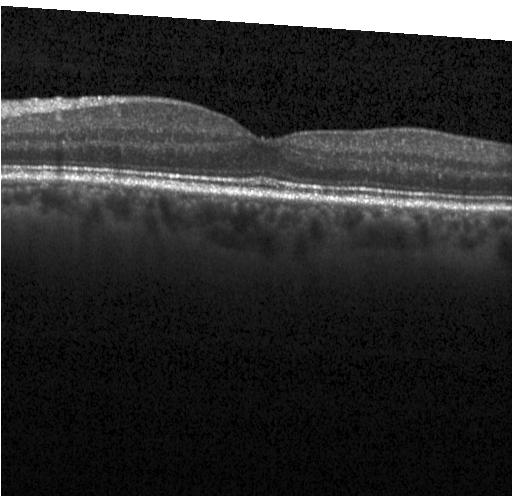

This B-scan demonstrates neither CNV, DME, nor drusen.